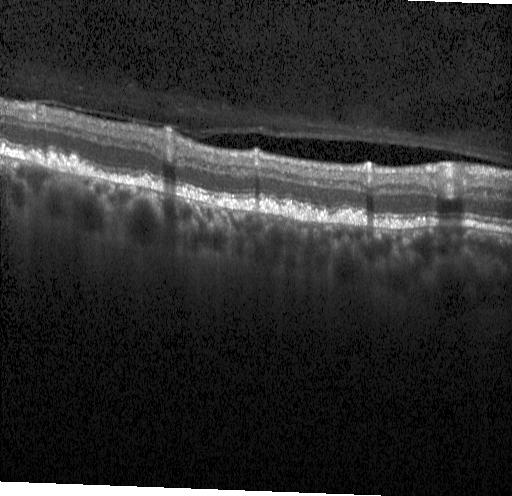 Impression: drusen.